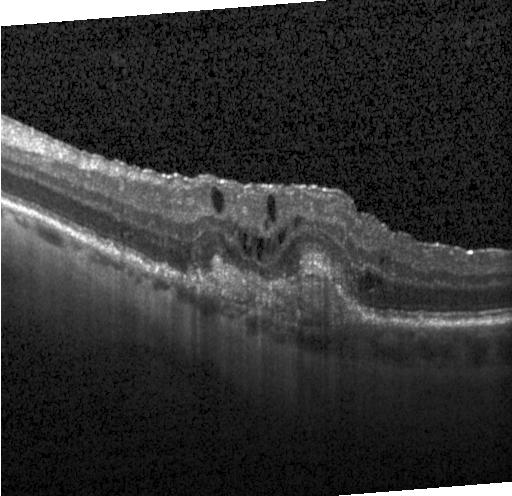 SD-OCT, Heidelberg Spectralis OCT system, OCT B-scan — Finding: a choroidal neovascular membrane.